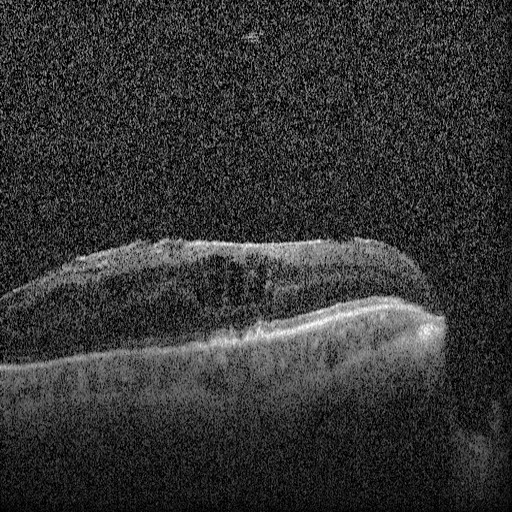
OCT line scan; Heidelberg Spectralis
Assessment: diabetic macular edema (DME).